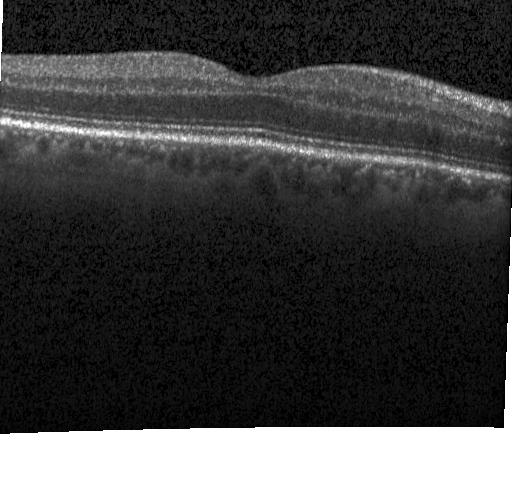

OCT line scan; acquired on a Heidelberg Spectralis — Finding: neither CNV, DME, nor drusen.